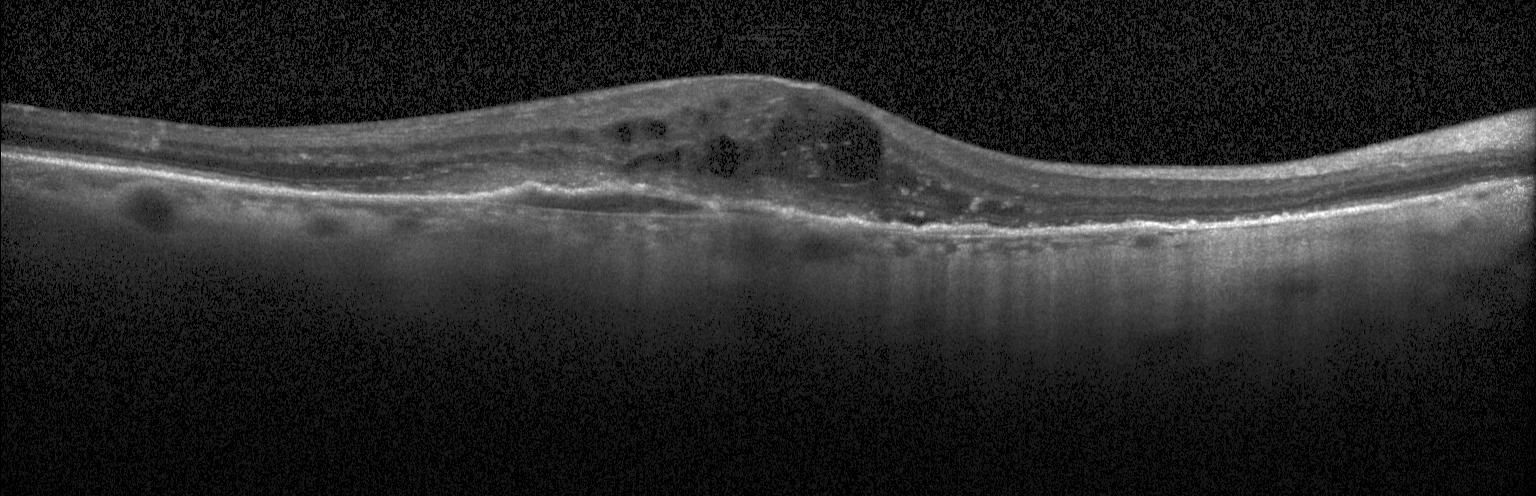
OCT B-scan · centered on the fovea · Heidelberg Spectralis OCT system · SD-OCT. Assessment: a choroidal neovascular membrane.